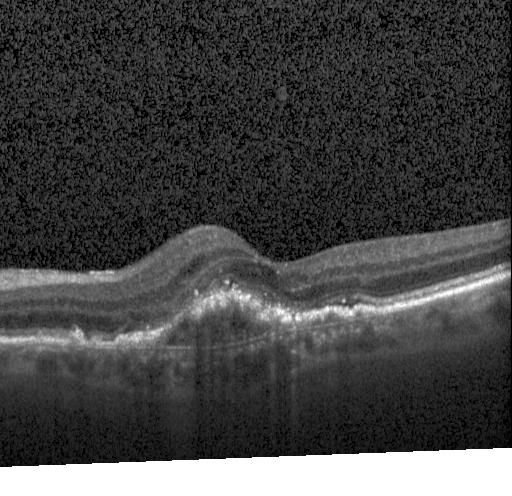 Optical coherence tomography scan; instrument: Heidelberg Spectralis; spectral-domain OCT
OCT finding: CNV.